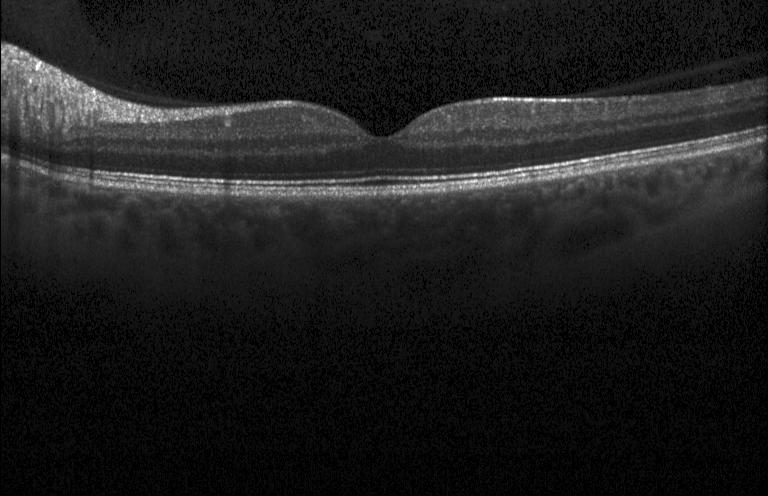 Optical coherence tomography B-scan; centered on the fovea; Heidelberg Spectralis; SD-OCT
Impression: neither choroidal neovascularization, diabetic macular edema, nor drusen.